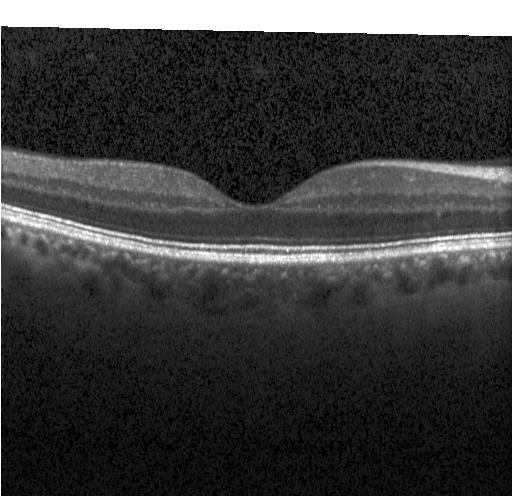 Spectral-domain optical coherence tomography. Retinal OCT B-scan. Heidelberg Spectralis OCT system.
Neither choroidal neovascularization, diabetic macular edema, nor drusen.